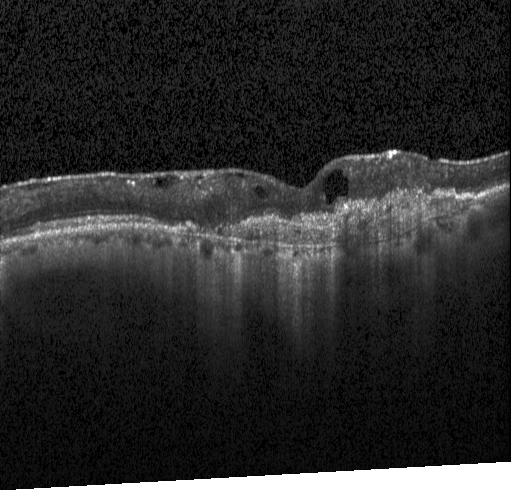 Optical coherence tomography scan.
OCT finding: a choroidal neovascular membrane.